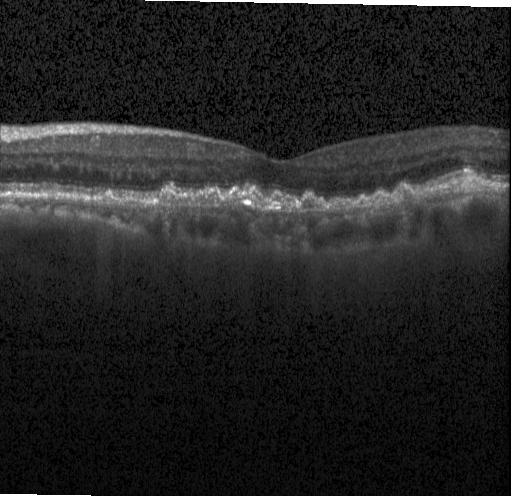

OCT B-scan showing CNV.